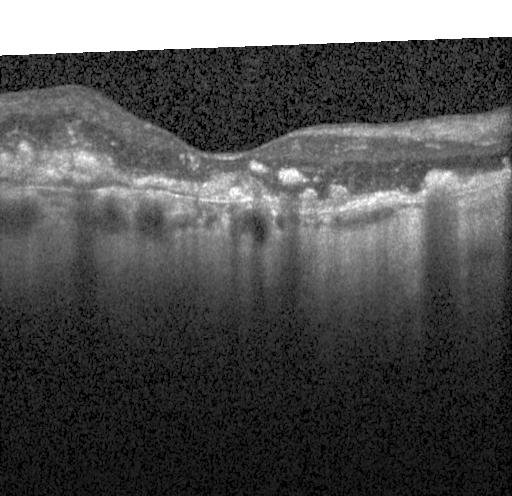
Retinal OCT B-scan, Heidelberg Spectralis OCT system, centered on the fovea, spectral-domain OCT. Dx: a choroidal neovascular membrane.